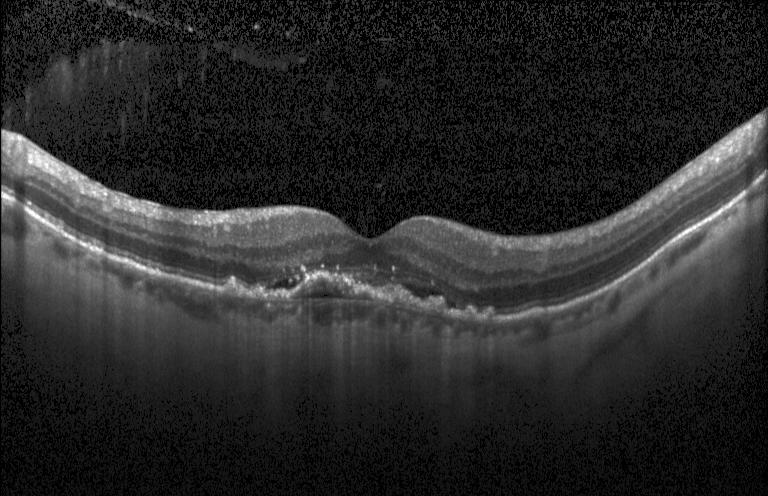
Optical coherence tomography scan. Spectral-domain OCT
Dx: choroidal neovascularization (CNV).